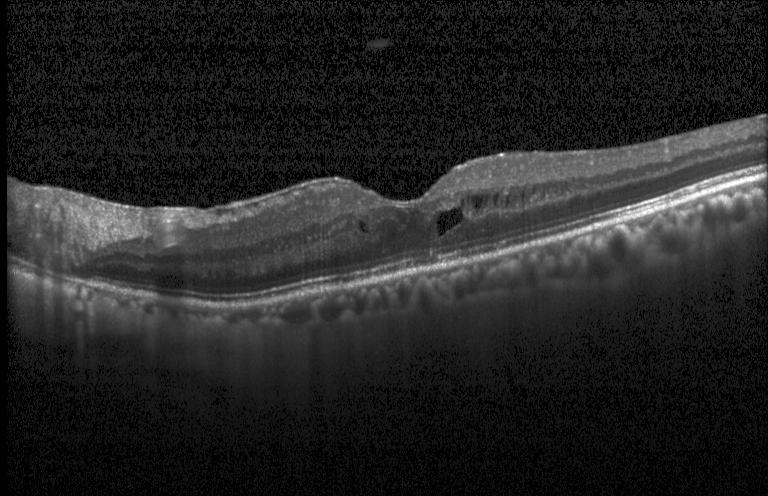 Retinal OCT B-scan · horizontal scan through the fovea · Heidelberg Spectralis · SD-OCT
Impression: DME.